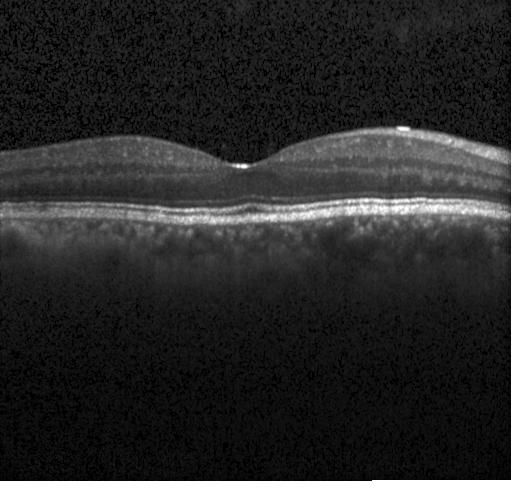
Macular scan · OCT B-scan · instrument: Heidelberg Spectralis.
Finding: neither choroidal neovascularization, diabetic macular edema, nor drusen.